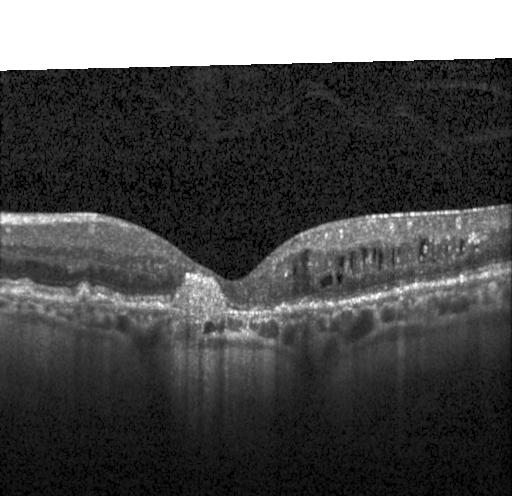

Spectral-domain OCT, macular scan, OCT B-scan, instrument: Heidelberg Spectralis.
Diagnosis: a choroidal neovascular membrane.